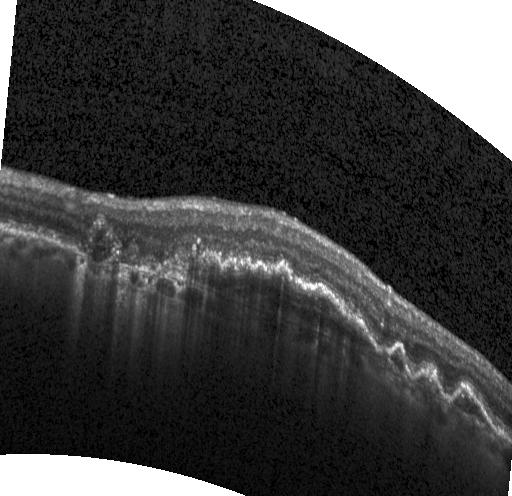

Impression: CNV.